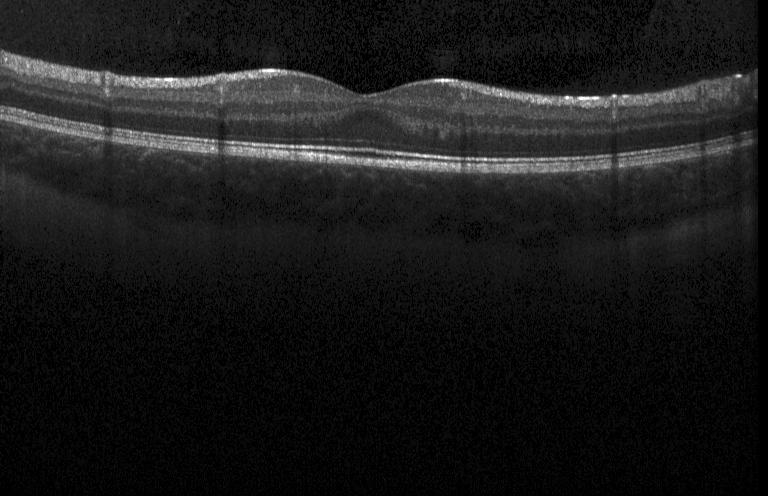

Finding: no choroidal neovascularization, no diabetic macular edema, and no drusen.